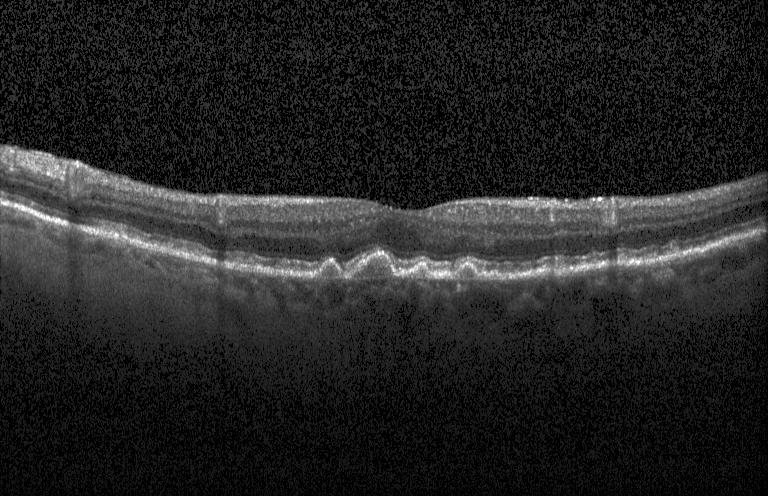

OCT B-scan showing sub-RPE drusenoid deposits.